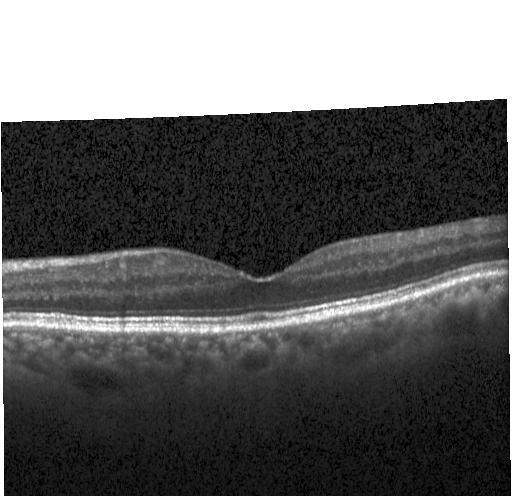
Impression: no evidence of choroidal neovascularization, diabetic macular edema, or drusen.